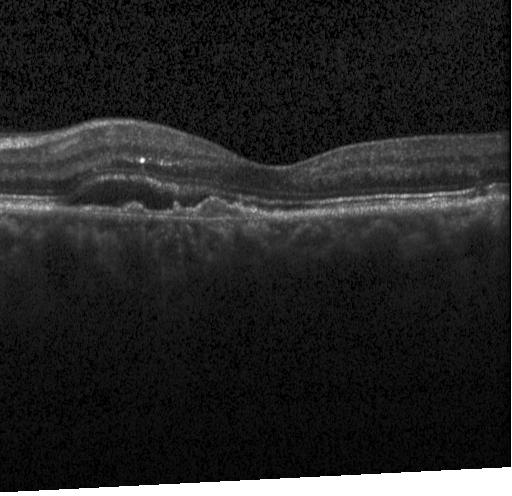
Optical coherence tomography B-scan — Diagnosis: CNV.